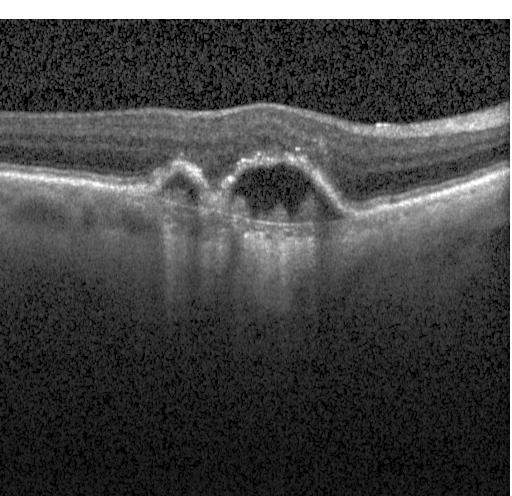 Optical coherence tomography scan; centered on the fovea. Finding: a choroidal neovascular membrane.